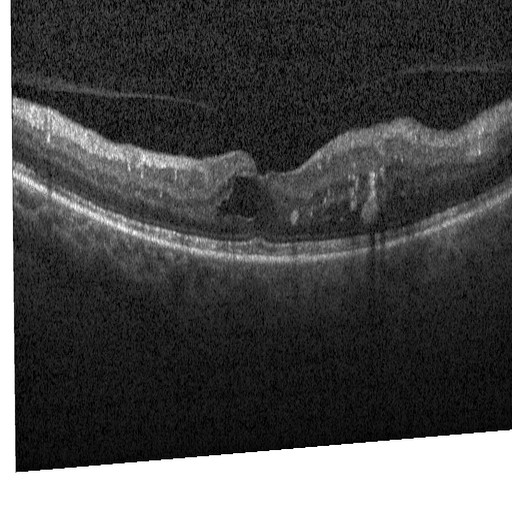

Macular scan · optical coherence tomography B-scan · SD-OCT. Macular OCT: diabetic macular edema.